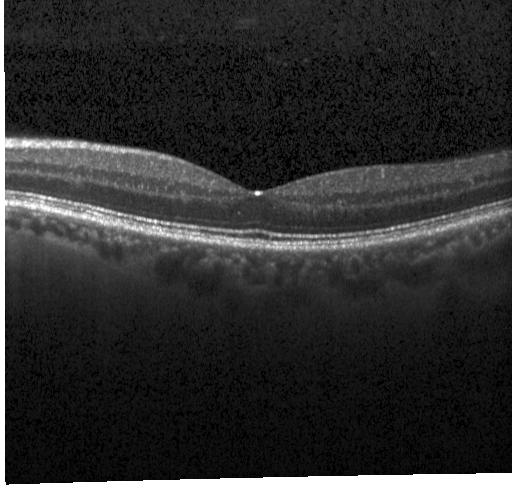
Optical coherence tomography B-scan, SD-OCT, Heidelberg Spectralis, horizontal scan through the fovea — Neither CNV, DME, nor drusen.